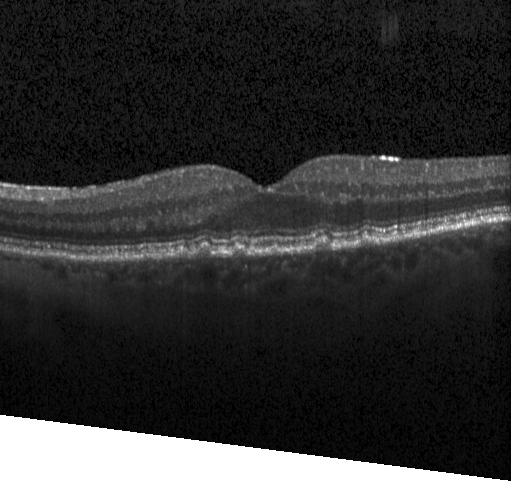
Multiple drusen.